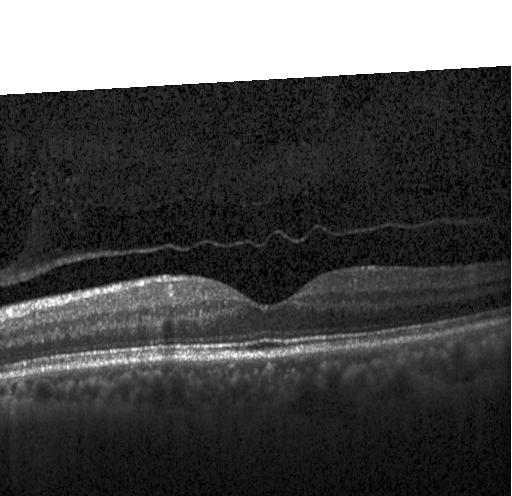
This B-scan demonstrates no choroidal neovascularization, no diabetic macular edema, and no drusen.